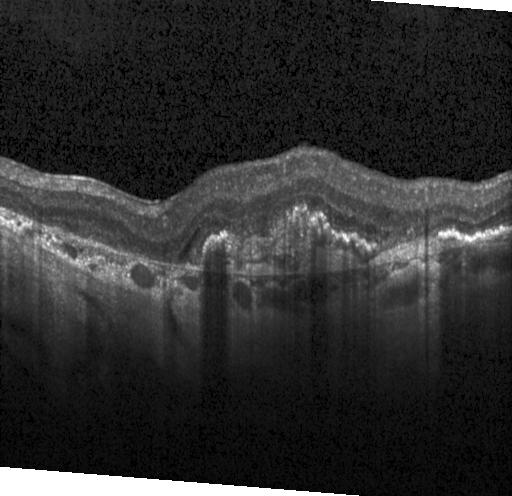
OCT B-scan showing a choroidal neovascular membrane.